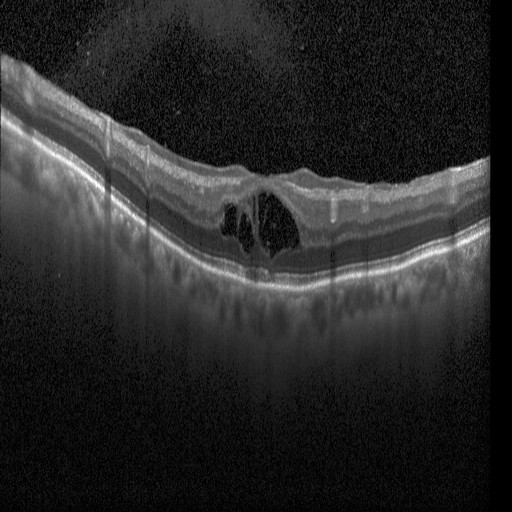 Optical coherence tomography B-scan, spectral-domain OCT. Dx: diabetic macular edema.